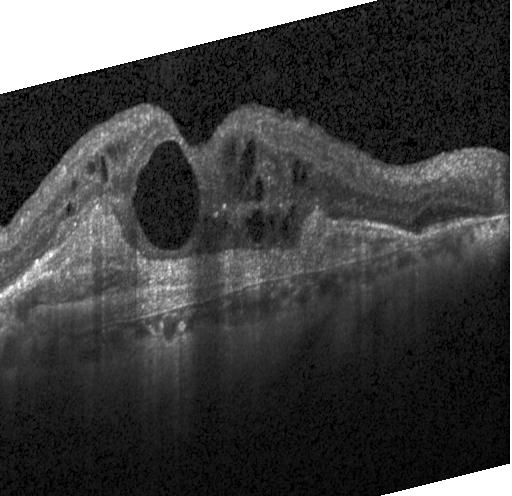

Diagnosis: CNV.